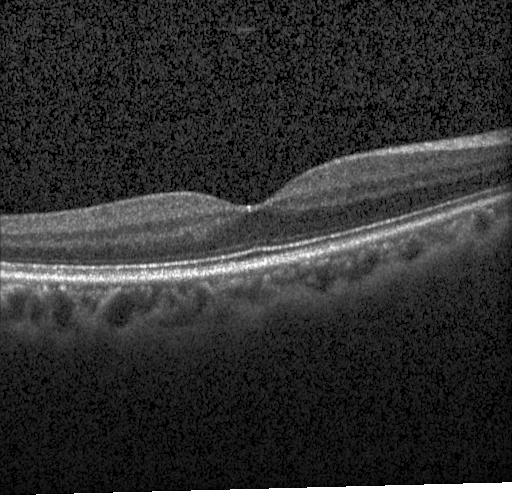

Retinal OCT cross-section. Heidelberg Spectralis OCT system. Assessment: neither choroidal neovascularization, diabetic macular edema, nor drusen.